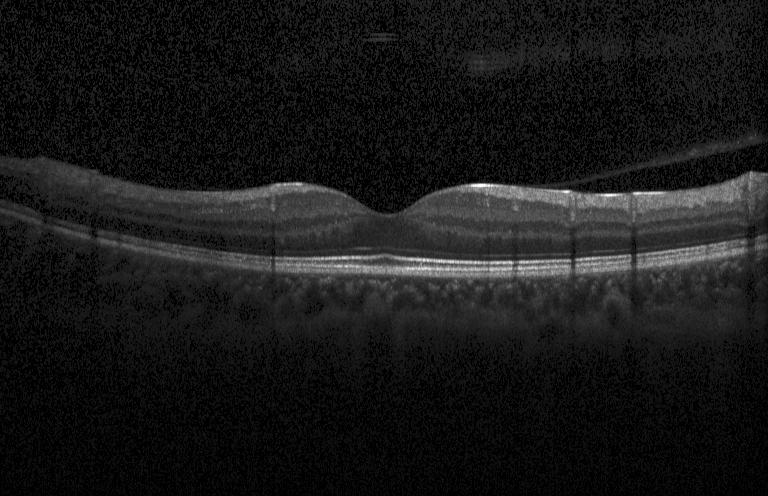

Macular OCT: no evidence of choroidal neovascularization, diabetic macular edema, or drusen.